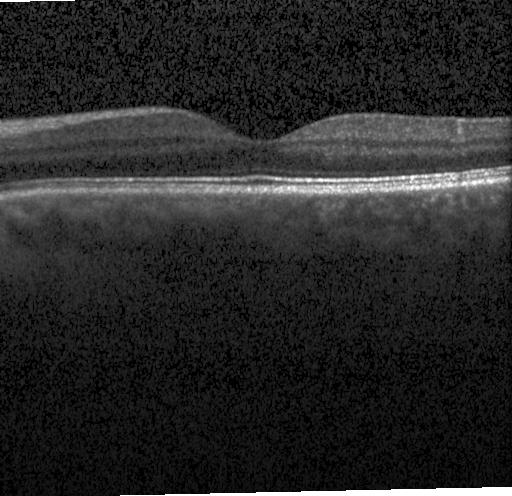
Diagnosis: no evidence of choroidal neovascularization, diabetic macular edema, or drusen.